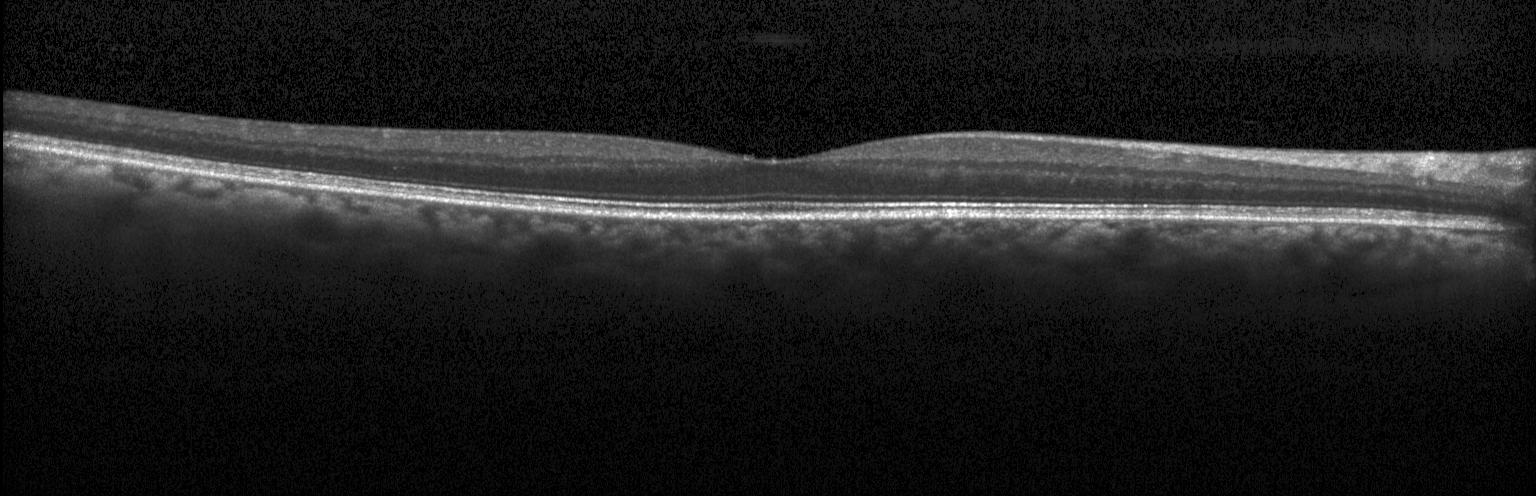

Diagnosis: neither choroidal neovascularization, diabetic macular edema, nor drusen.